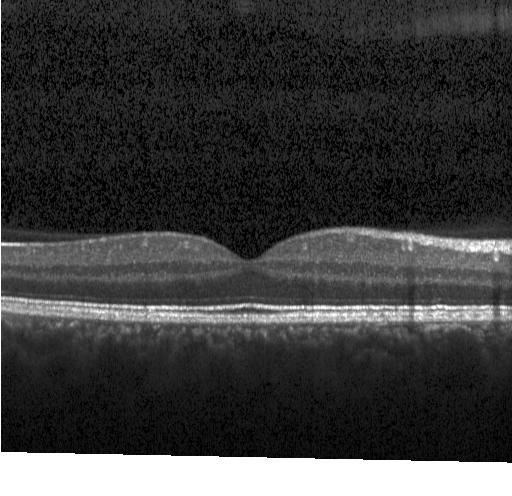 Horizontal scan through the fovea. Instrument: Heidelberg Spectralis. Optical coherence tomography B-scan — OCT finding: neither choroidal neovascularization, diabetic macular edema, nor drusen.